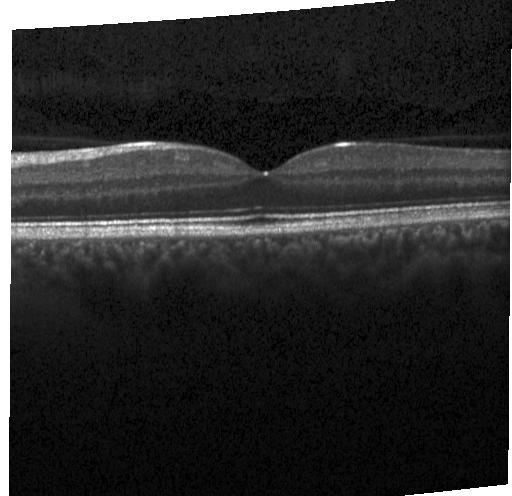
OCT B-scan. Impression: no evidence of CNV, DME, or drusen.